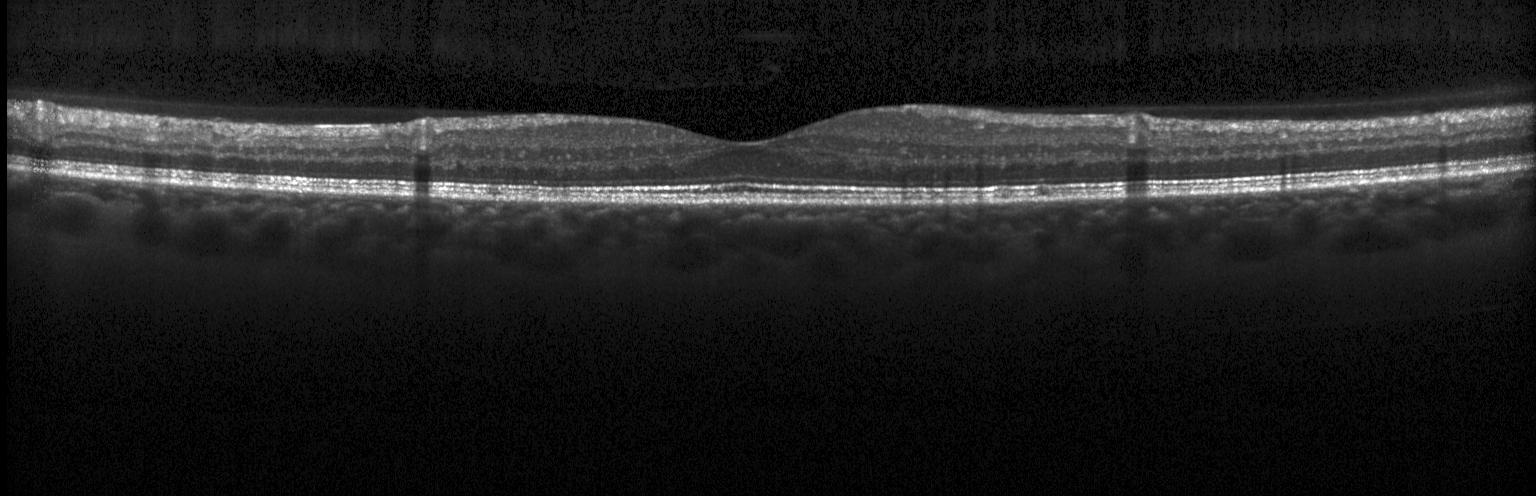

OCT line scan.
Neither choroidal neovascularization, diabetic macular edema, nor drusen.